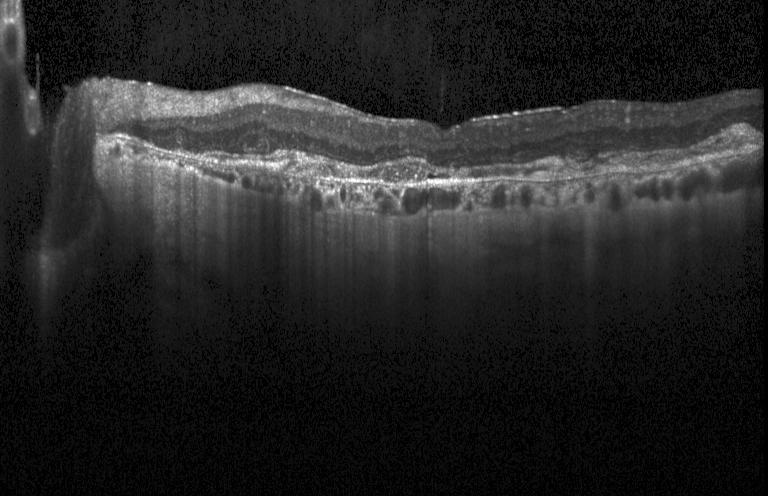
Optical coherence tomography B-scan, horizontal scan through the fovea, instrument: Heidelberg Spectralis
The scan shows CNV.